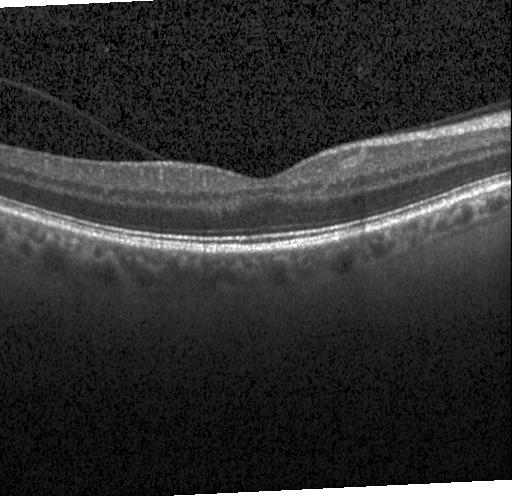

Optical coherence tomography B-scan, spectral-domain OCT, Heidelberg Spectralis, horizontal scan through the fovea. No CNV, no DME, and no drusen.